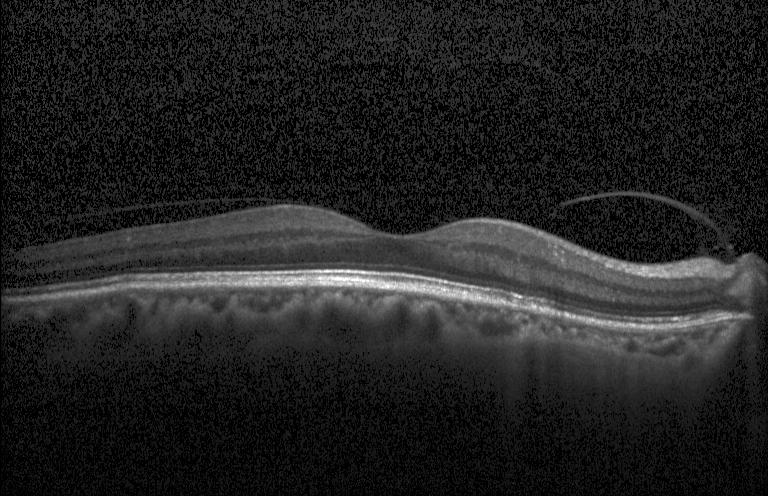
Through the macula. Spectral-domain OCT. Retinal OCT cross-section. Heidelberg Spectralis OCT system. Finding: neither CNV, DME, nor drusen.